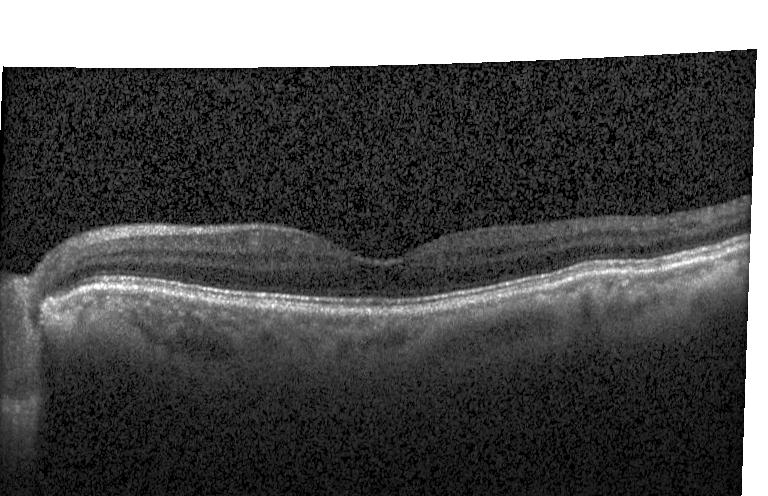

Spectral-domain OCT. OCT line scan — Neither CNV, DME, nor drusen.